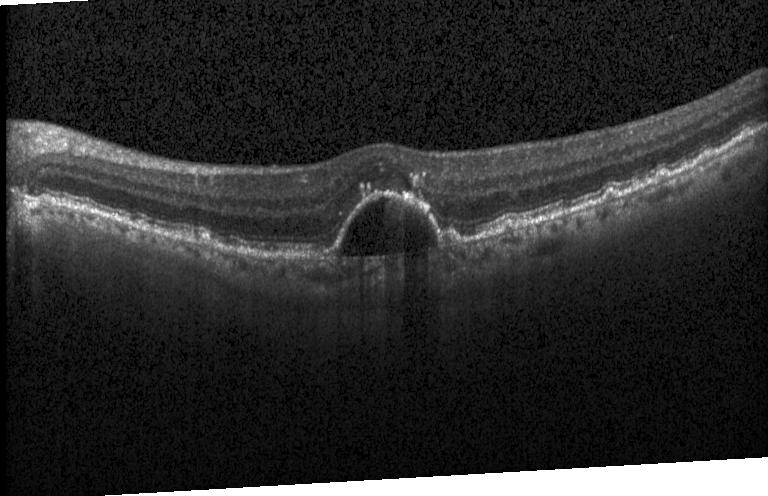 SD-OCT, acquired on a Heidelberg Spectralis, OCT line scan — Assessment: a choroidal neovascular membrane.